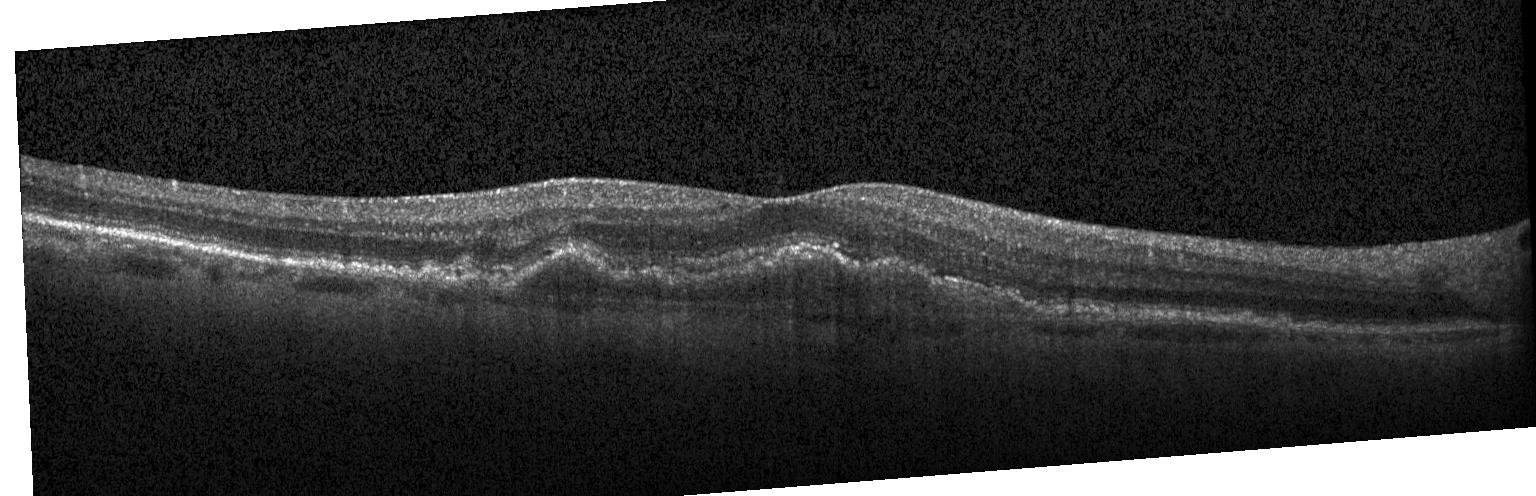 OCT B-scan · instrument: Heidelberg Spectralis
Assessment: a choroidal neovascular membrane.